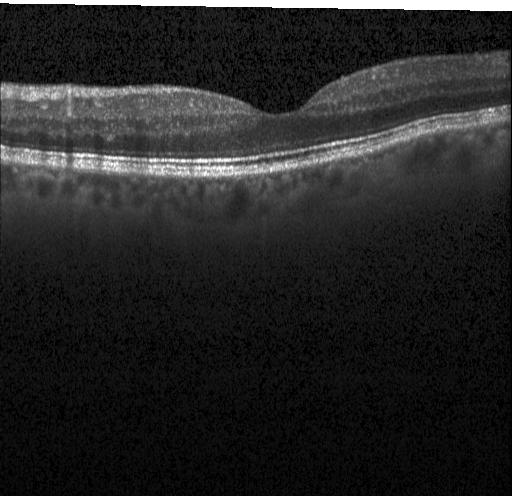 Fovea-centered. Spectral-domain optical coherence tomography. Heidelberg Spectralis OCT system. Optical coherence tomography scan.
This B-scan demonstrates no evidence of choroidal neovascularization, diabetic macular edema, or drusen.